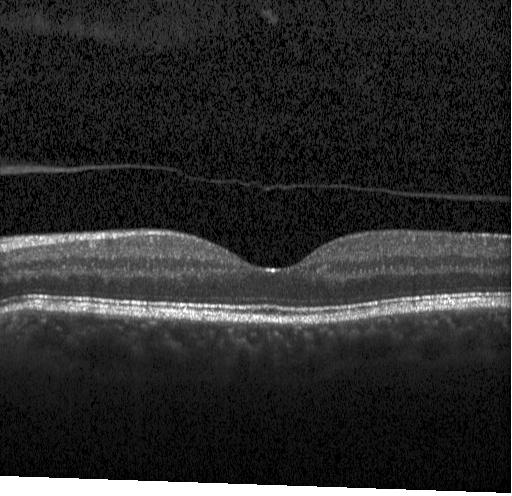 Spectral-domain OCT B-scan: no evidence of CNV, DME, or drusen.